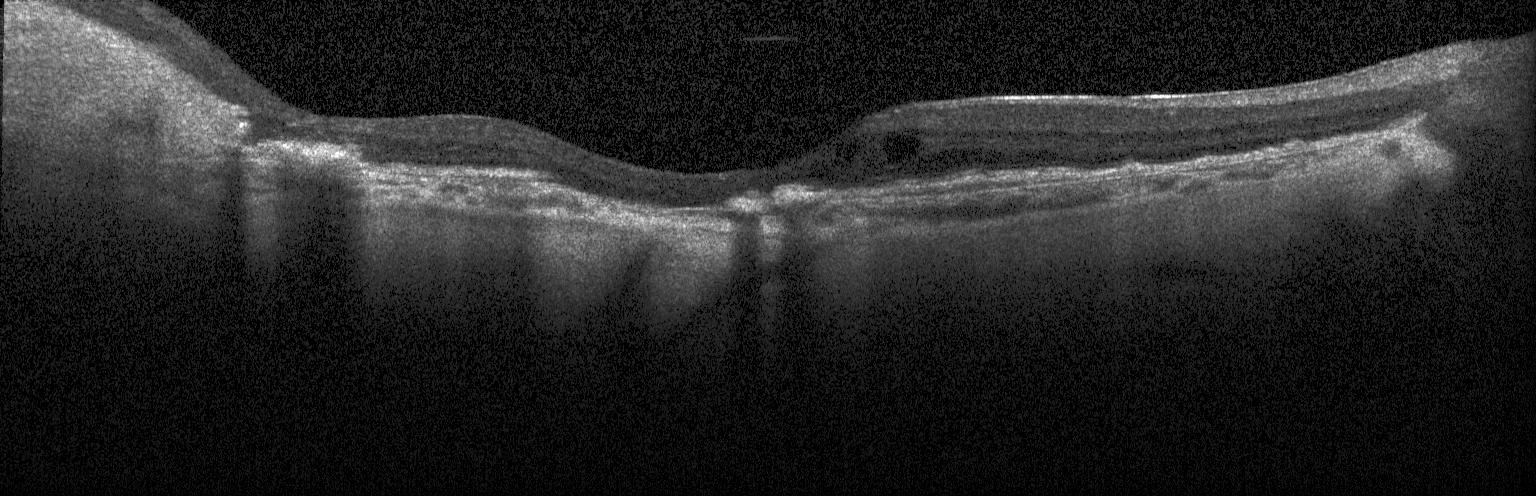

Optical coherence tomography B-scan · macular scan · spectral-domain OCT — A choroidal neovascular membrane.